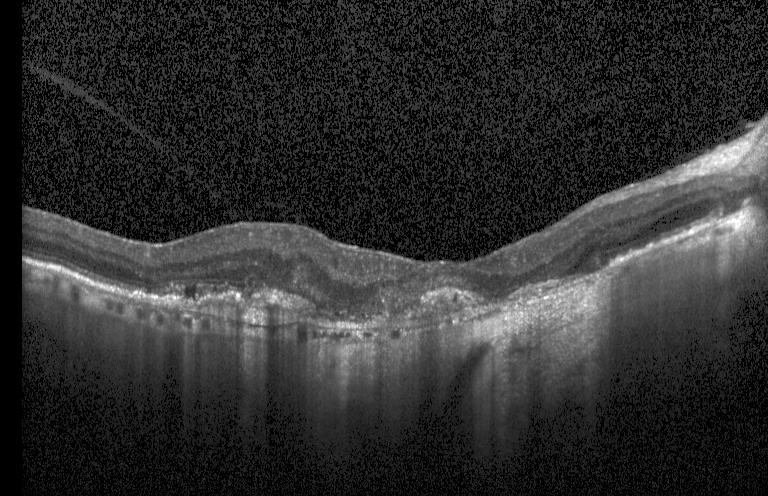

Impression: a choroidal neovascular membrane.